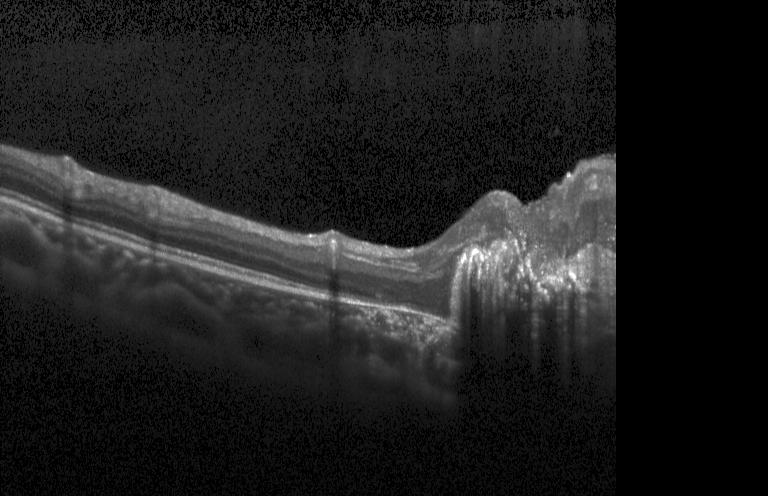 Retinal OCT B-scan. Diagnosis: choroidal neovascularization.